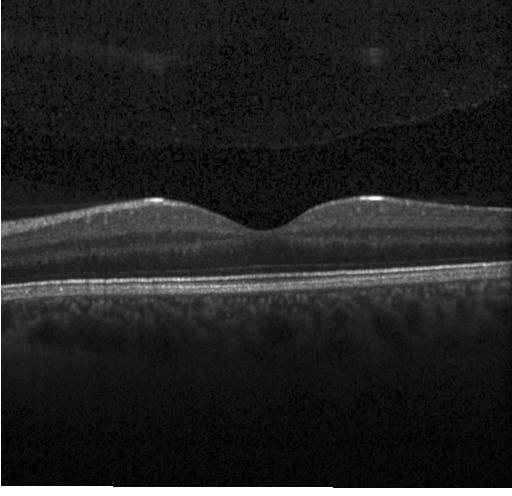
Retinal OCT B-scan
Assessment: no choroidal neovascularization, no diabetic macular edema, and no drusen.